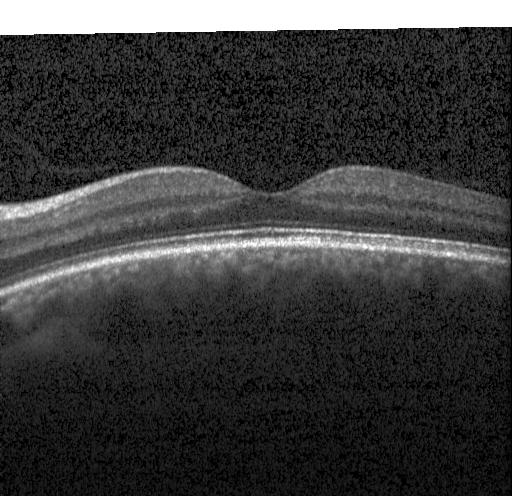 Finding: no CNV, no DME, and no drusen.